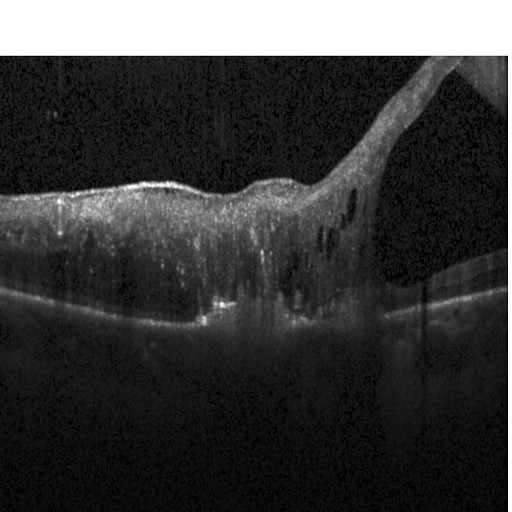 Retinal OCT B-scan. Impression: DME.